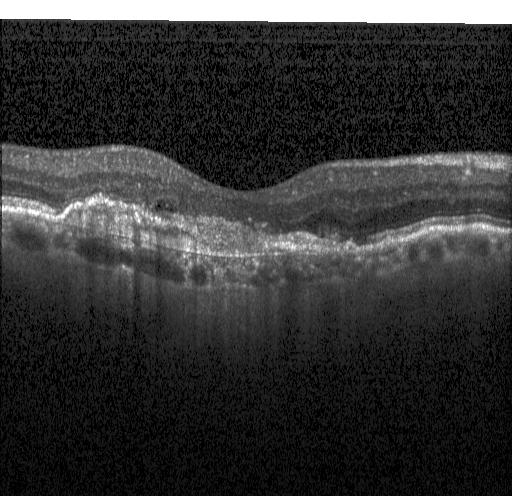 Macular scan; retinal OCT cross-section — Macular OCT: a choroidal neovascular membrane.